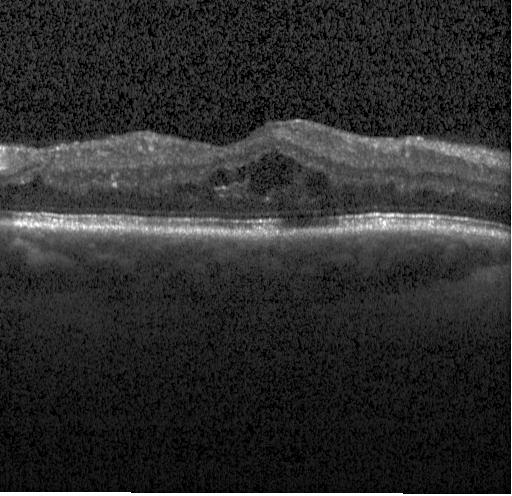

Spectral-domain OCT, retinal OCT B-scan
Dx: DME.